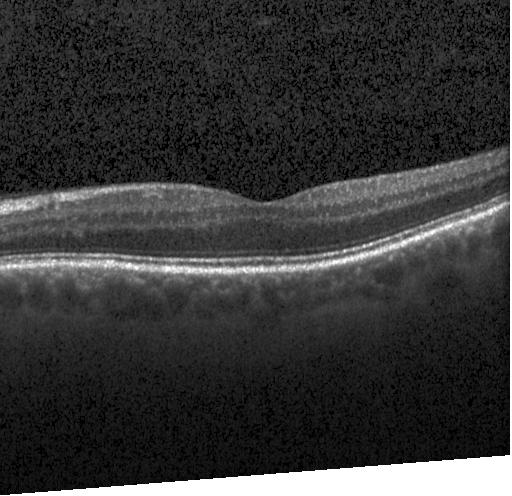 Retinal OCT B-scan; macular scan; instrument: Heidelberg Spectralis; SD-OCT — Impression: no evidence of choroidal neovascularization, diabetic macular edema, or drusen.